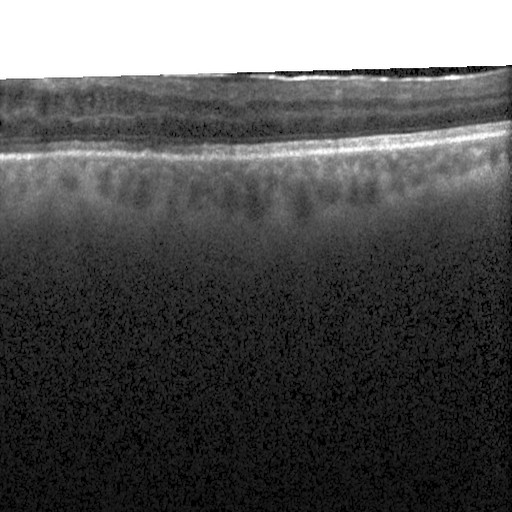
Dx: diabetic macular edema.